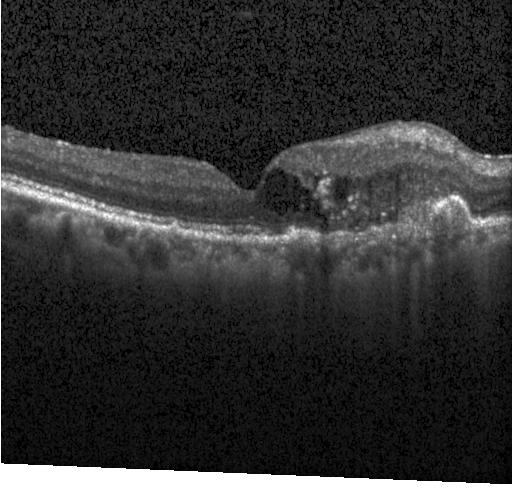
Optical coherence tomography scan
Diagnosis: choroidal neovascularization.